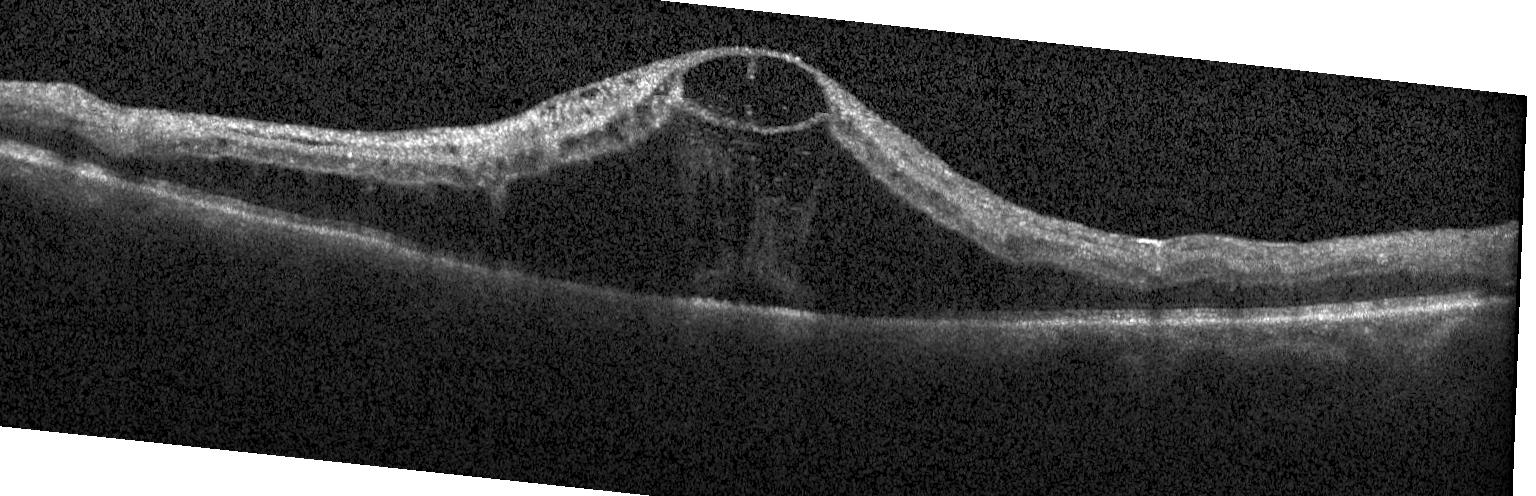 OCT line scan. Fovea-centered. Finding: diabetic macular edema (DME).